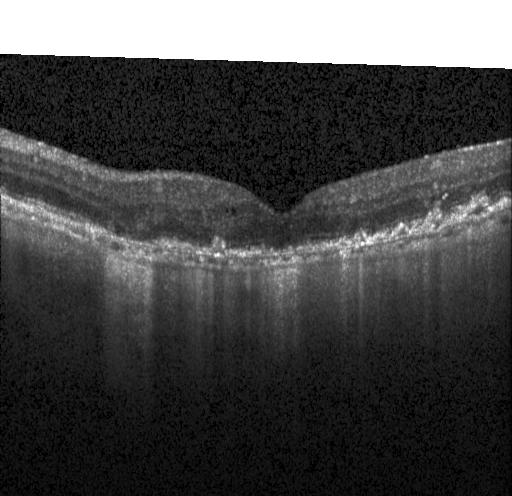
Assessment: a choroidal neovascular membrane.